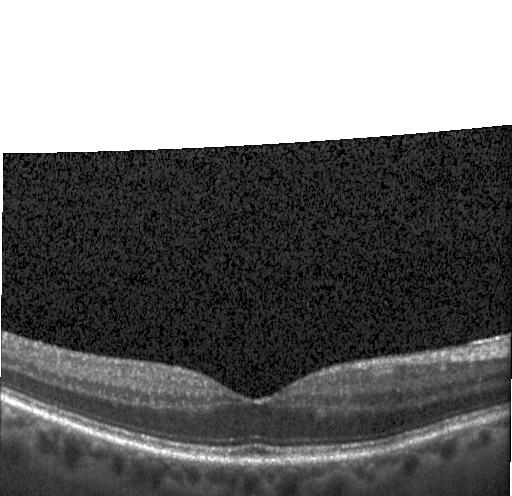

SD-OCT; optical coherence tomography scan
Impression: no evidence of choroidal neovascularization, diabetic macular edema, or drusen.